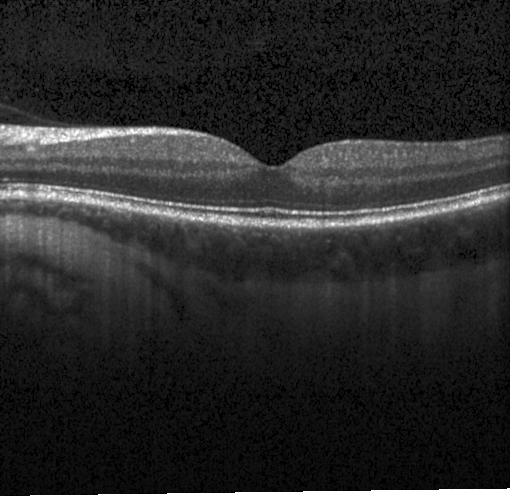
OCT B-scan — Assessment: no evidence of CNV, DME, or drusen.